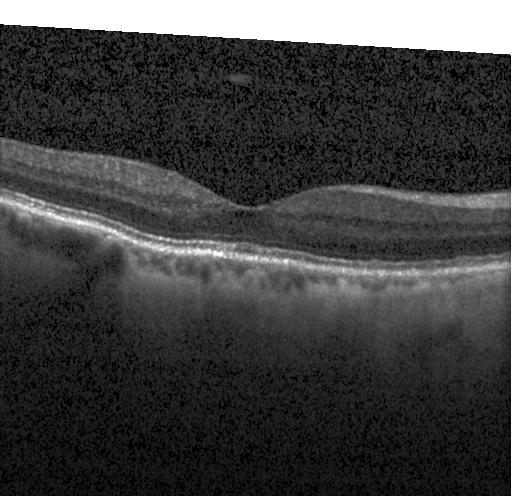 Instrument: Heidelberg Spectralis; retinal OCT cross-section; fovea-centered — Assessment: no choroidal neovascularization, diabetic macular edema, or drusen.